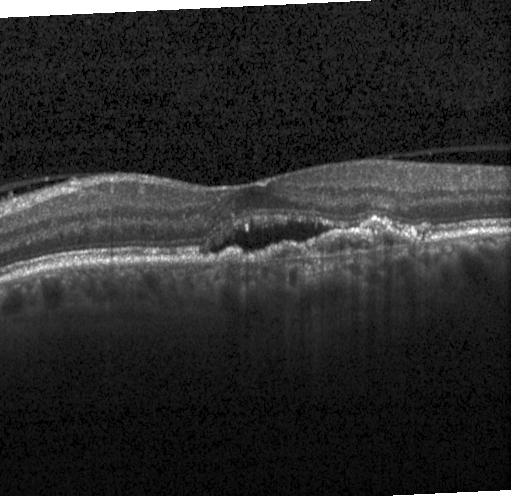 Optical coherence tomography B-scan. Heidelberg Spectralis. Horizontal scan through the fovea. Spectral-domain OCT.
The scan shows choroidal neovascularization (CNV).